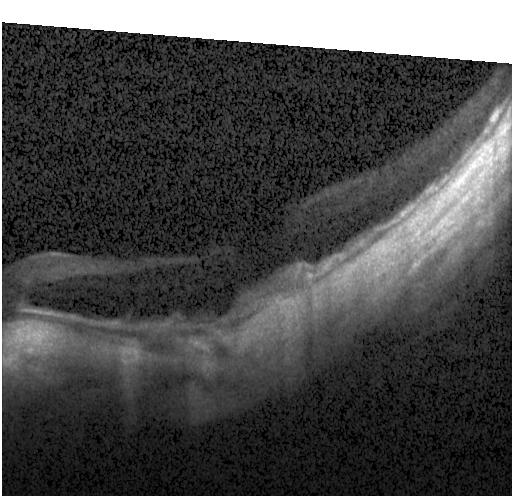

Dx: choroidal neovascularization.